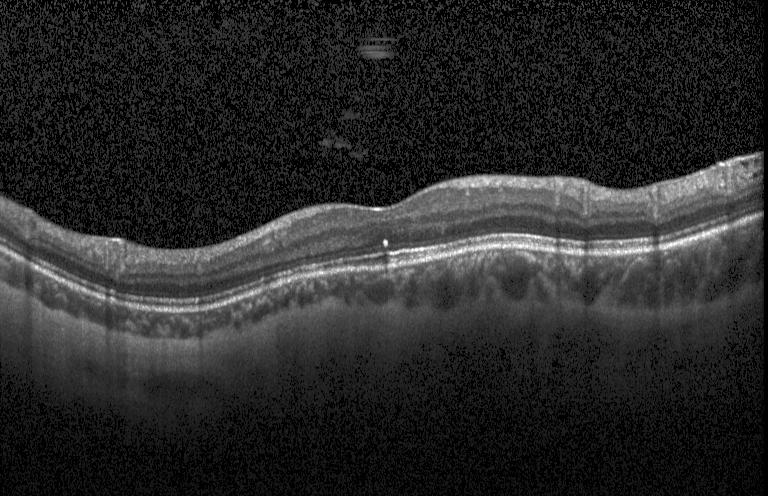

Fovea-centered. Heidelberg Spectralis. Spectral-domain optical coherence tomography. Retinal OCT cross-section. Diagnosis: no choroidal neovascularization, no diabetic macular edema, and no drusen.